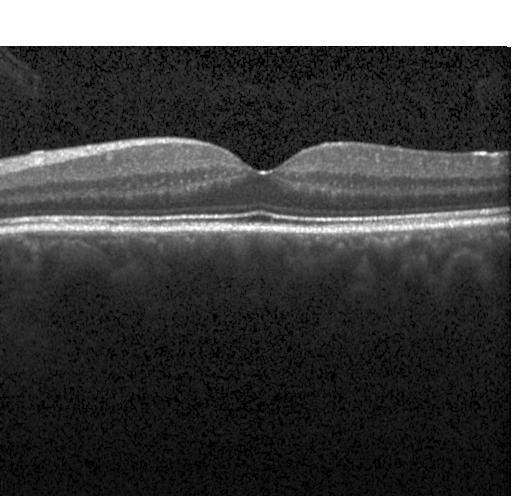 Centered on the fovea · optical coherence tomography scan.
OCT finding: no choroidal neovascularization, no diabetic macular edema, and no drusen.